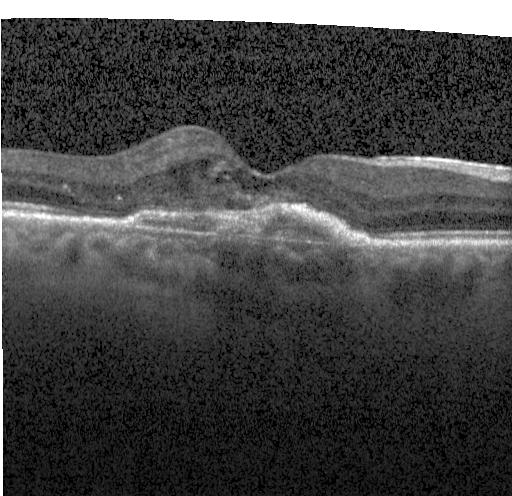 Retinal OCT B-scan; spectral-domain OCT.
This B-scan demonstrates a choroidal neovascular membrane.